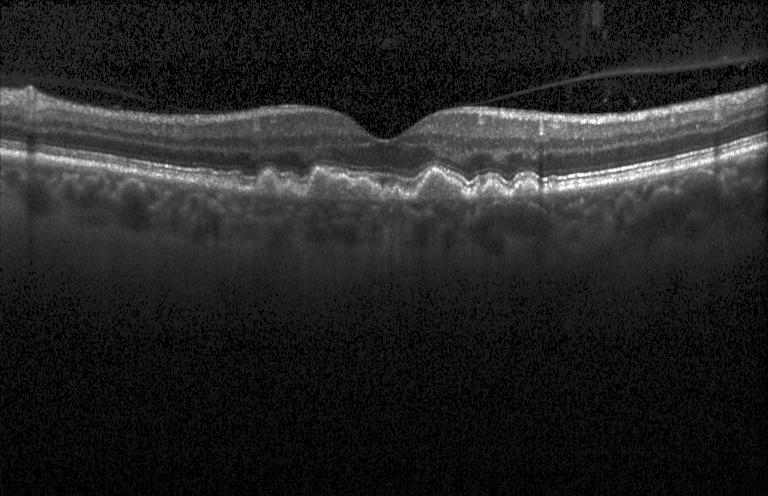 Retinal OCT B-scan; acquired on a Heidelberg Spectralis. Finding: drusen.